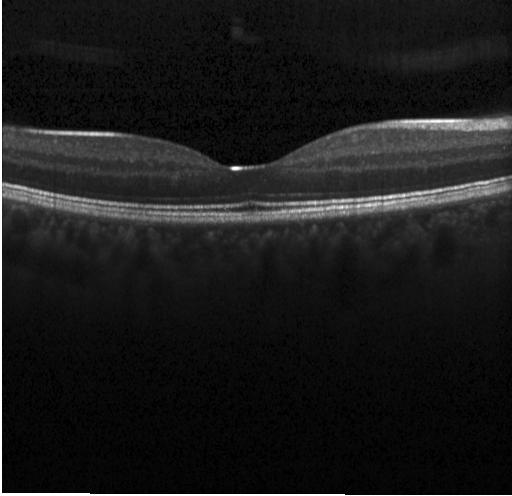 Retinal OCT cross-section showing no choroidal neovascularization, diabetic macular edema, or drusen.